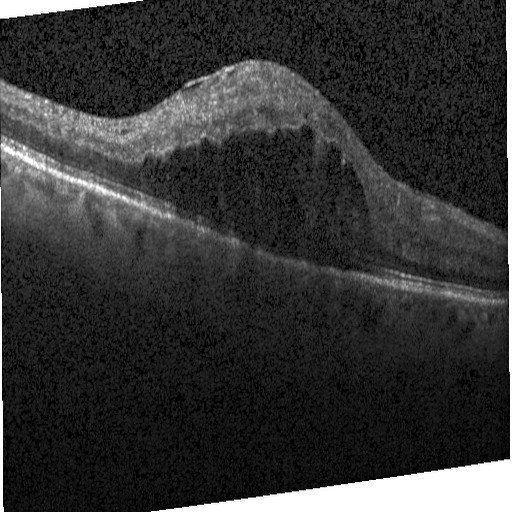
Acquired on a Heidelberg Spectralis. Macular scan. Retinal OCT cross-section. OCT finding: diabetic macular edema (DME).